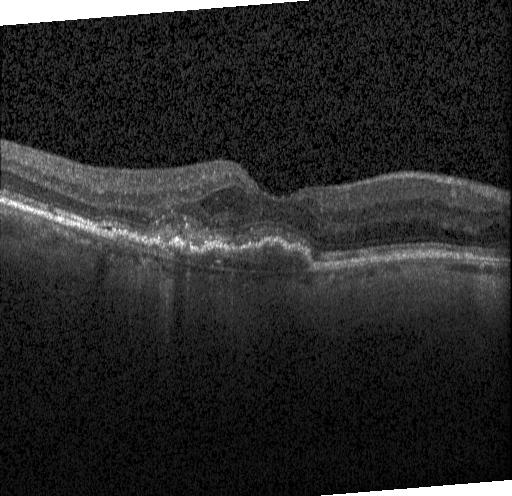

OCT scan showing choroidal neovascularization (CNV).